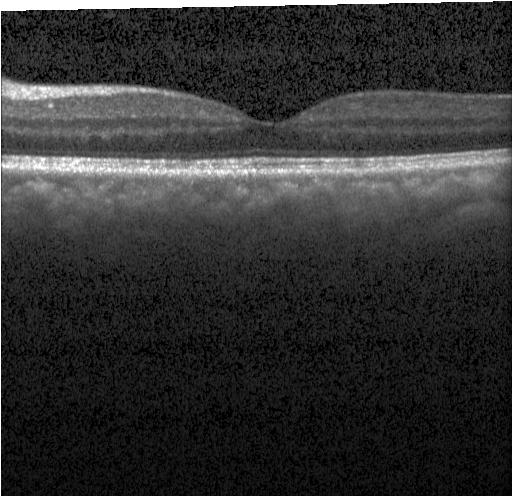

Macular scan. Retinal OCT cross-section. Instrument: Heidelberg Spectralis. Spectral-domain OCT. Macular OCT: no CNV, DME, or drusen.